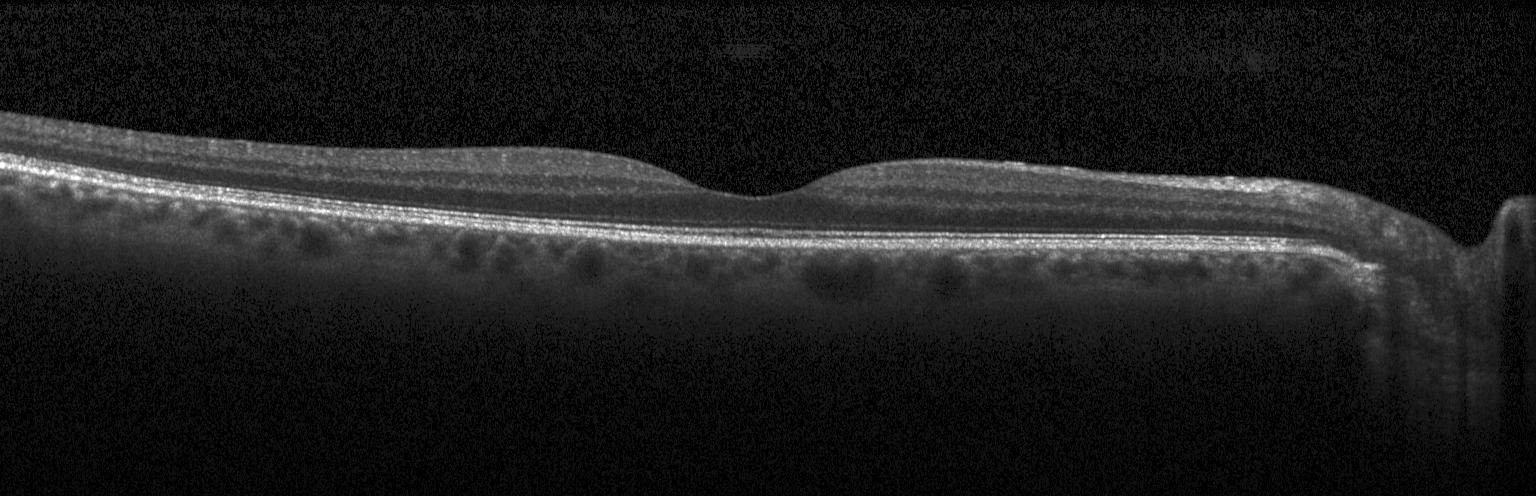

Macular scan · Heidelberg Spectralis OCT system · optical coherence tomography B-scan · spectral-domain optical coherence tomography — No choroidal neovascularization, diabetic macular edema, or drusen.